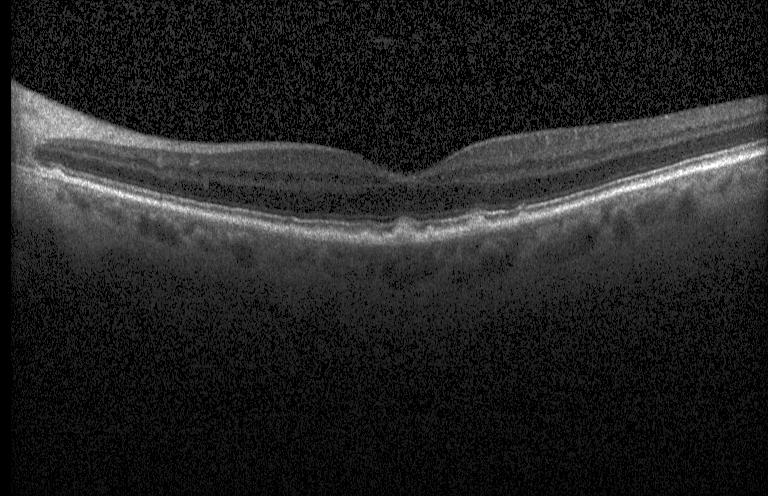

Optical coherence tomography B-scan · Heidelberg Spectralis OCT system
Assessment: multiple drusen.